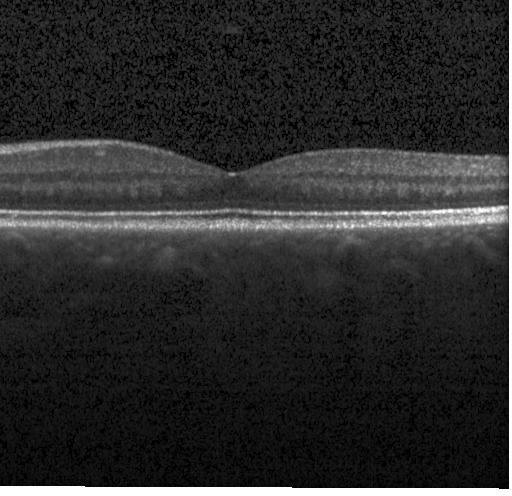

Fovea-centered; optical coherence tomography B-scan — Diagnosis: neither CNV, DME, nor drusen.